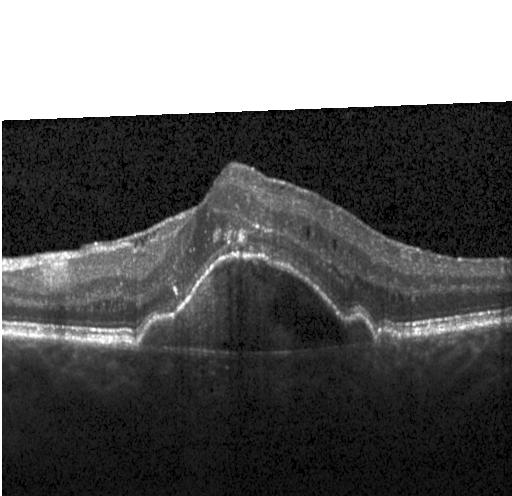
Retinal OCT cross-section showing choroidal neovascularization (CNV).